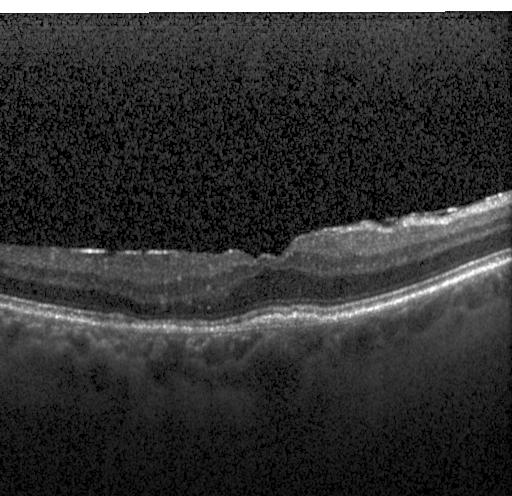

Horizontal scan through the fovea. Retinal OCT cross-section. Assessment: choroidal neovascularization.